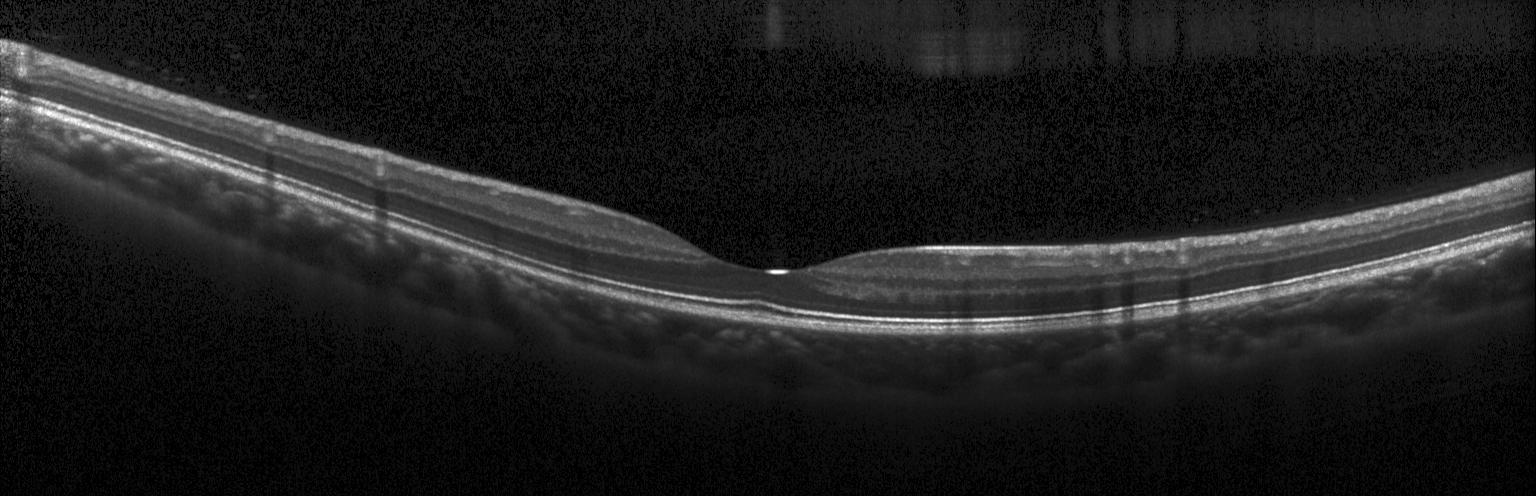

OCT line scan
Dx: no CNV, DME, or drusen.